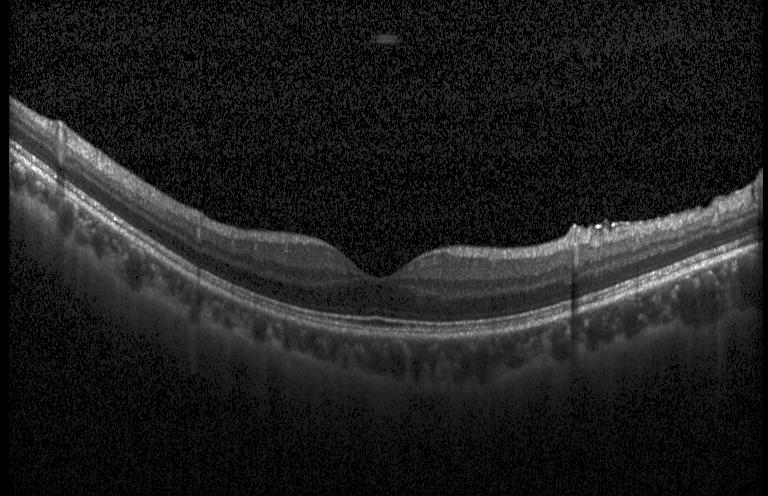
Macular scan, retinal OCT B-scan.
OCT finding: neither CNV, DME, nor drusen.